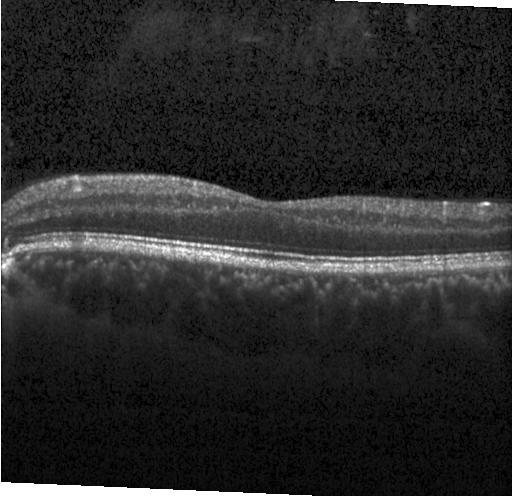

Dx: no choroidal neovascularization, no diabetic macular edema, and no drusen.